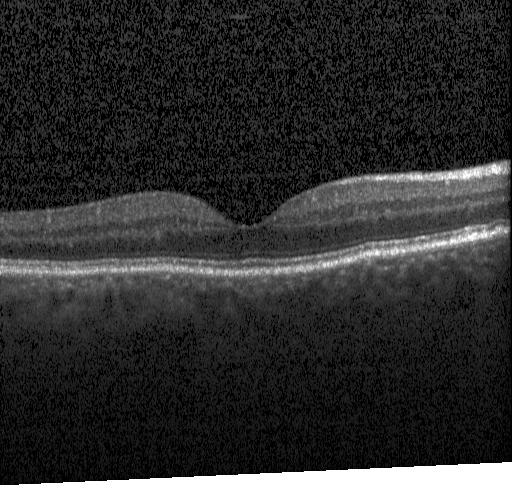

Optical coherence tomography B-scan; horizontal scan through the fovea; spectral-domain optical coherence tomography.
The scan shows no CNV, DME, or drusen.